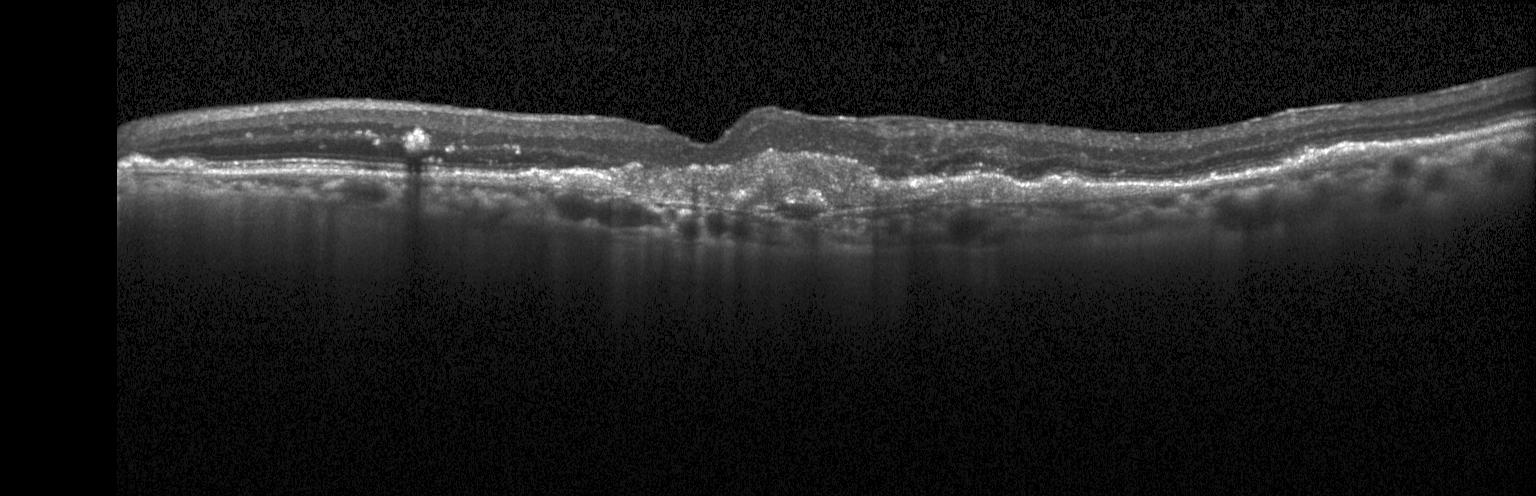

Fovea-centered, spectral-domain optical coherence tomography, optical coherence tomography B-scan, Heidelberg Spectralis OCT system
A choroidal neovascular membrane.